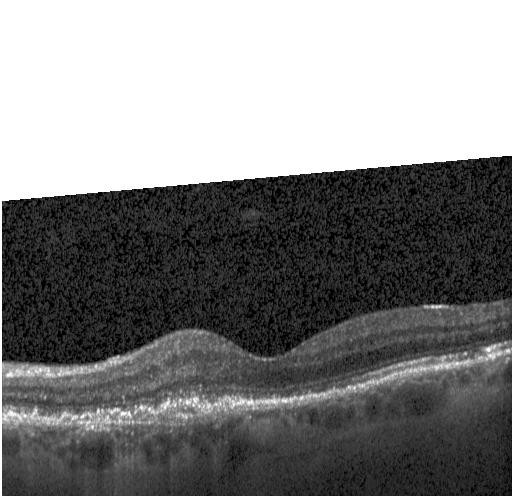

Impression: a choroidal neovascular membrane.